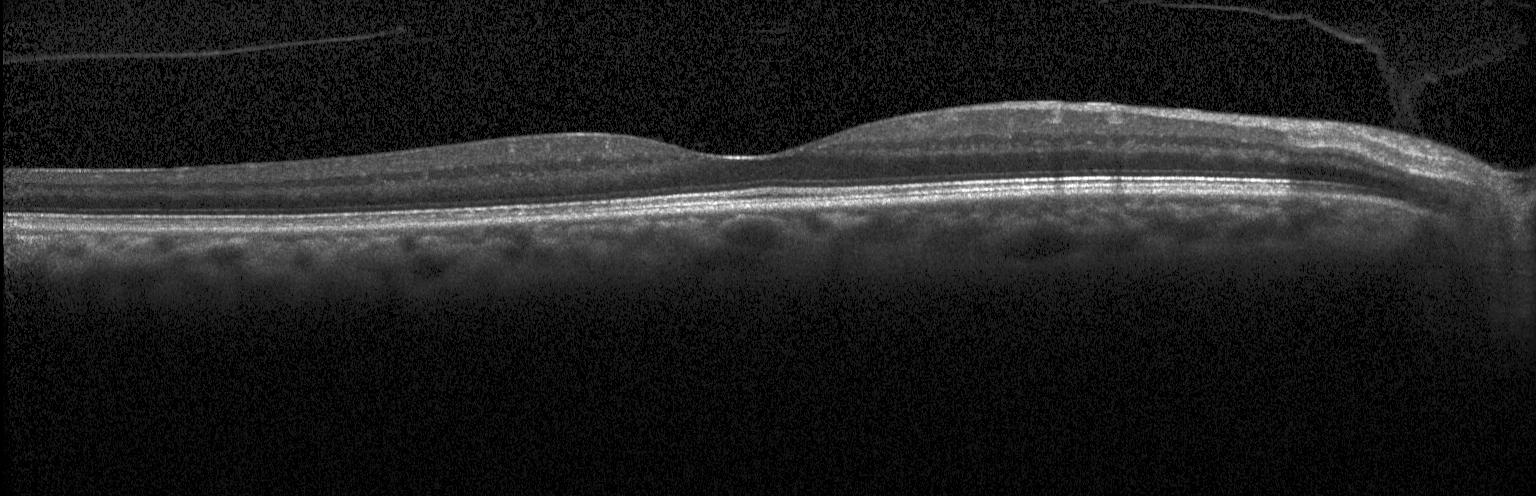

The scan shows neither CNV, DME, nor drusen.